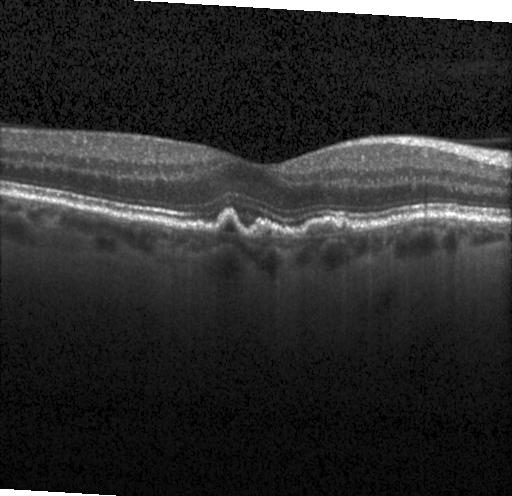
Impression: drusen.